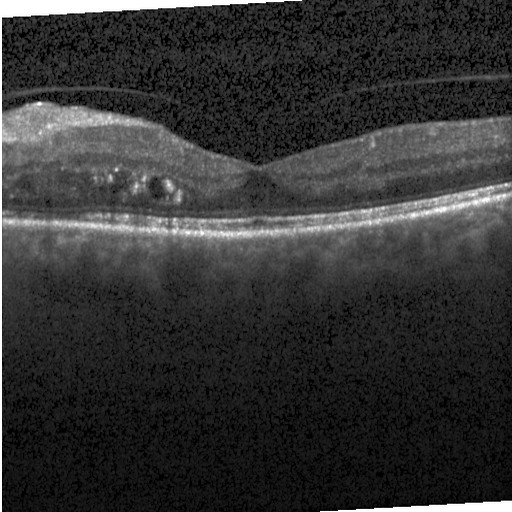
Diabetic macular edema (DME).